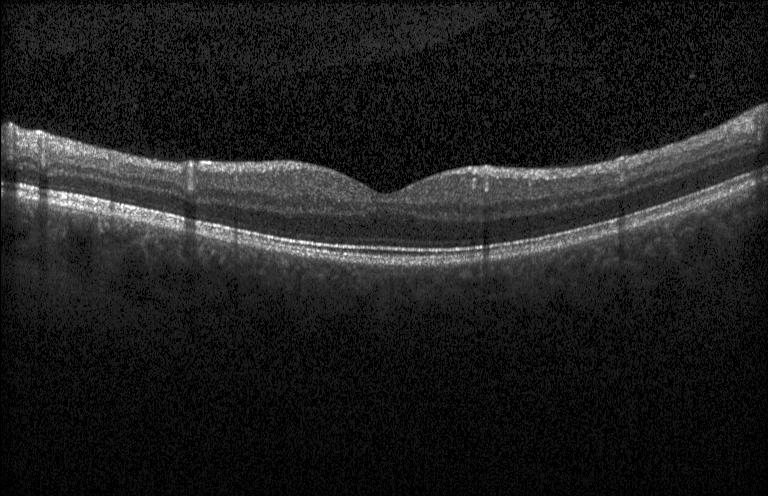 Instrument: Heidelberg Spectralis; fovea-centered; optical coherence tomography scan
Assessment: neither choroidal neovascularization, diabetic macular edema, nor drusen.